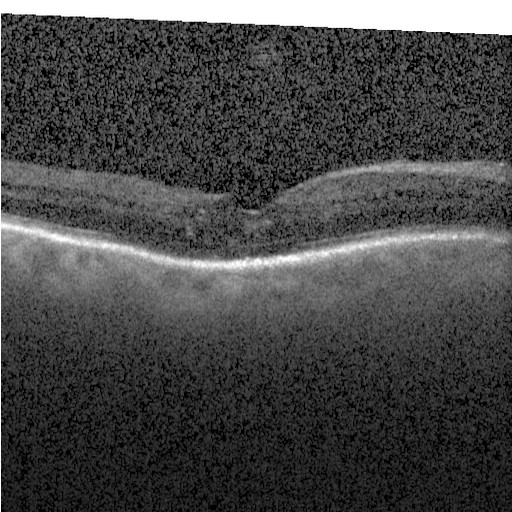 OCT B-scan showing diabetic macular edema.